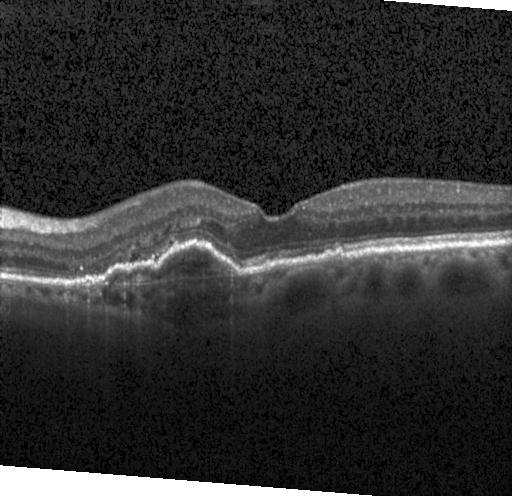
Optical coherence tomography B-scan, macular scan
Assessment: choroidal neovascularization (CNV).